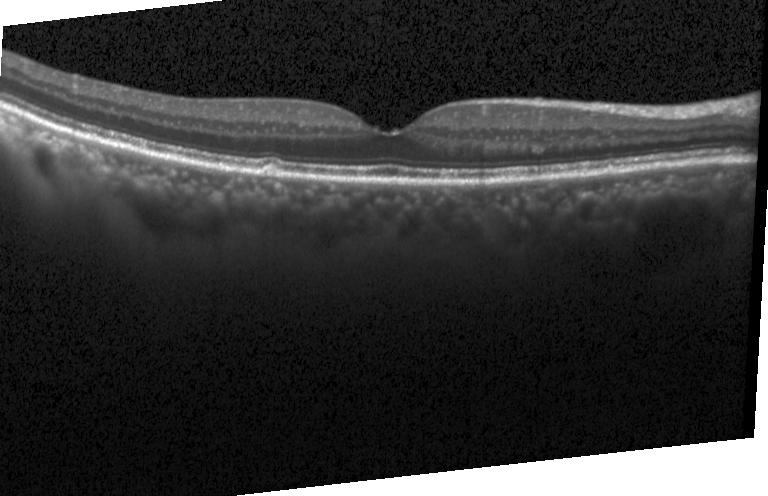
Horizontal scan through the fovea. Optical coherence tomography B-scan. Heidelberg Spectralis OCT system — OCT finding: multiple drusen.